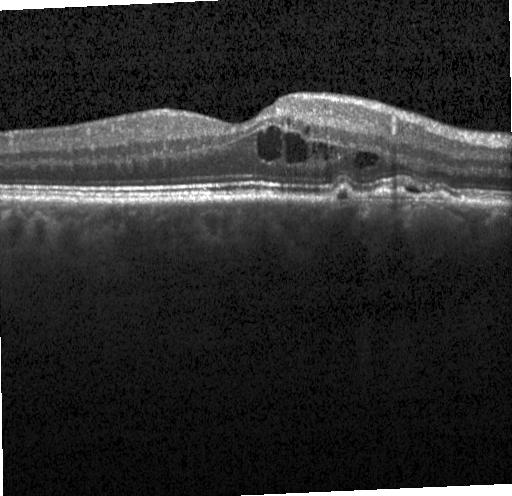 Optical coherence tomography scan. Finding: choroidal neovascularization.